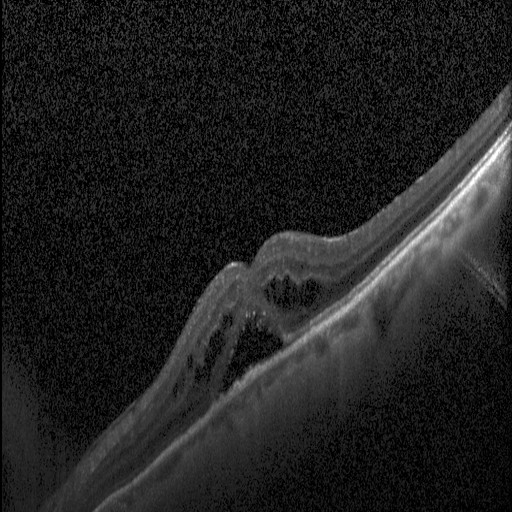
SD-OCT. Optical coherence tomography scan. Fovea-centered. Instrument: Heidelberg Spectralis
Diagnosis: DME.